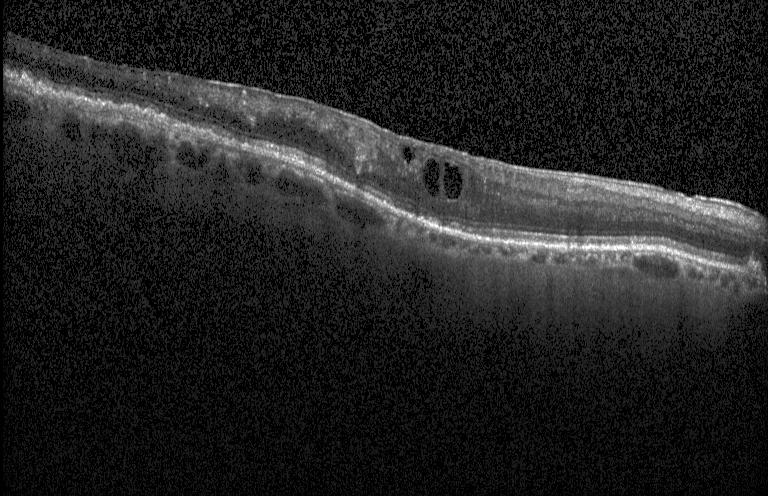

Horizontal scan through the fovea. Optical coherence tomography scan
Macular OCT: a choroidal neovascular membrane.